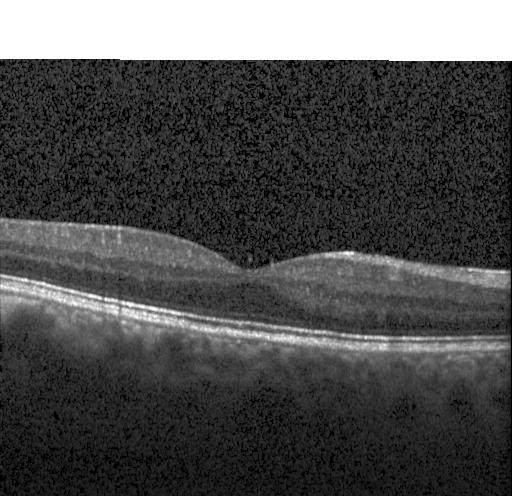
Diagnosis: neither CNV, DME, nor drusen.